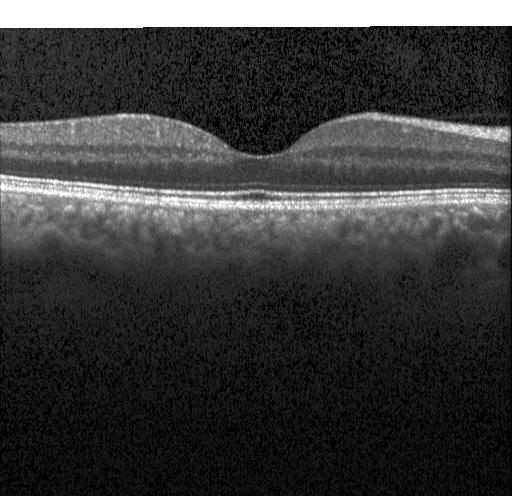 The scan shows no choroidal neovascularization, diabetic macular edema, or drusen.